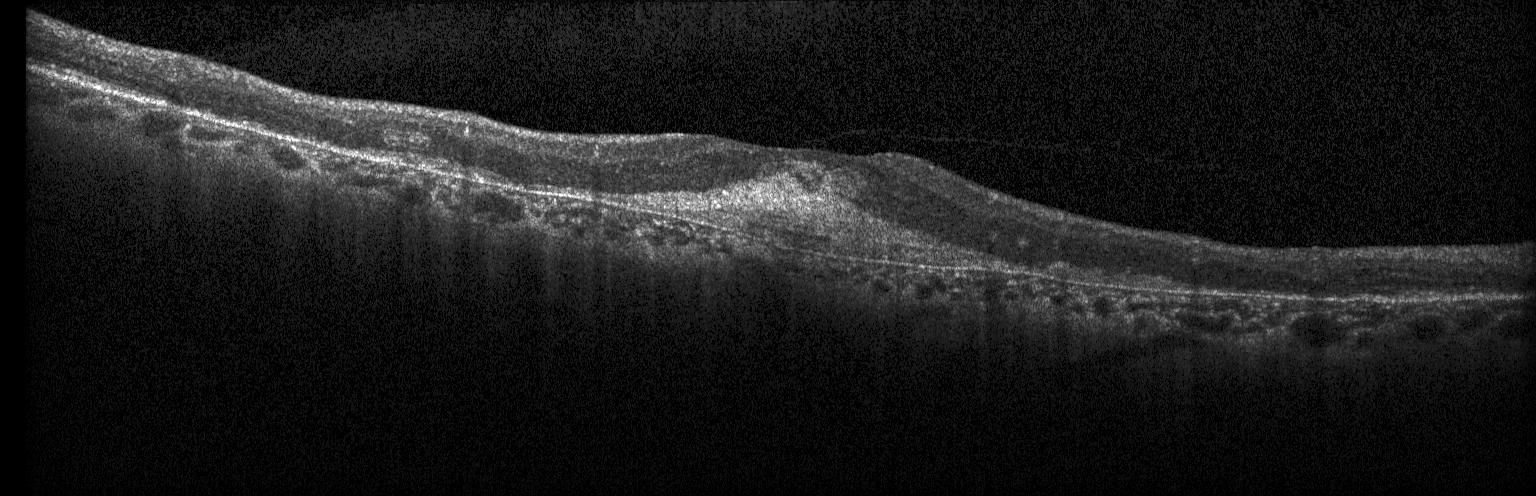

OCT B-scan.
Macular OCT: a choroidal neovascular membrane.